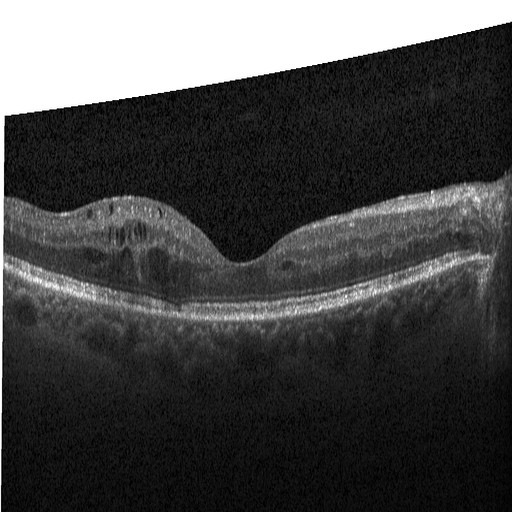 Macular OCT: diabetic macular edema.